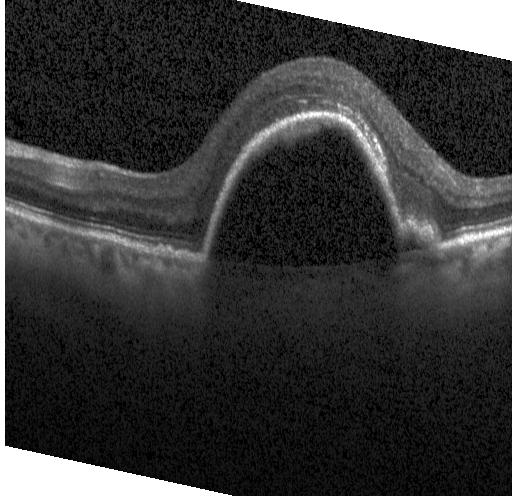
Retinal OCT cross-section, SD-OCT. Finding: choroidal neovascularization.